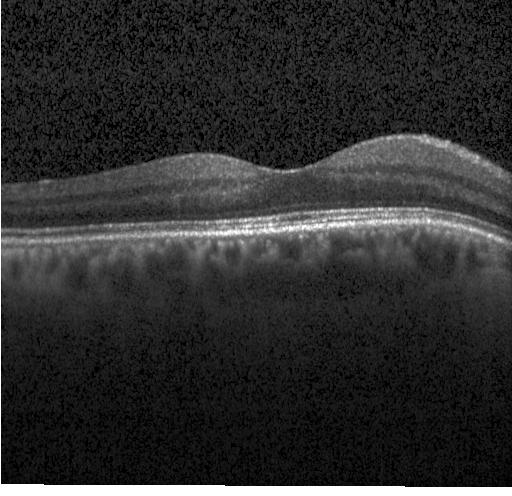 Retinal OCT cross-section
Finding: no CNV, no DME, and no drusen.